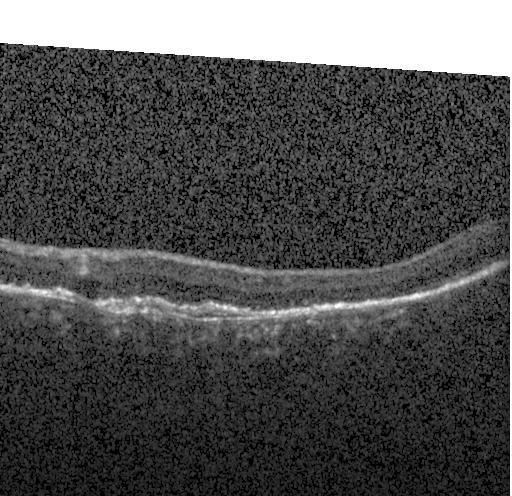
Optical coherence tomography B-scan. A choroidal neovascular membrane.